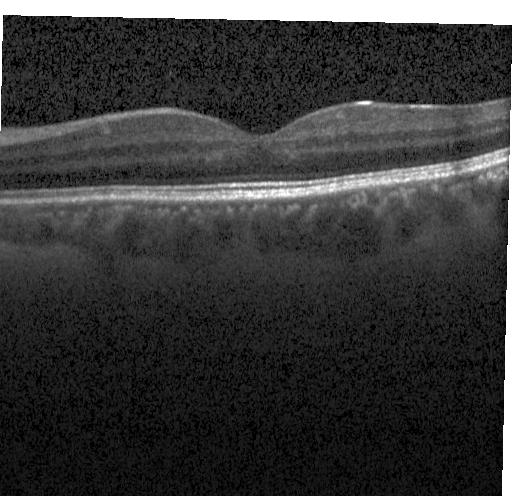 Spectral-domain OCT · retinal OCT B-scan
This B-scan demonstrates neither CNV, DME, nor drusen.